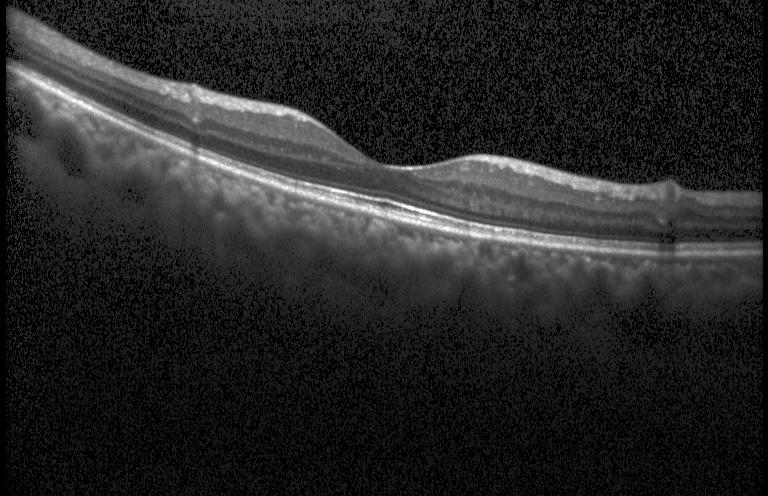 Optical coherence tomography scan. OCT finding: no CNV, DME, or drusen.